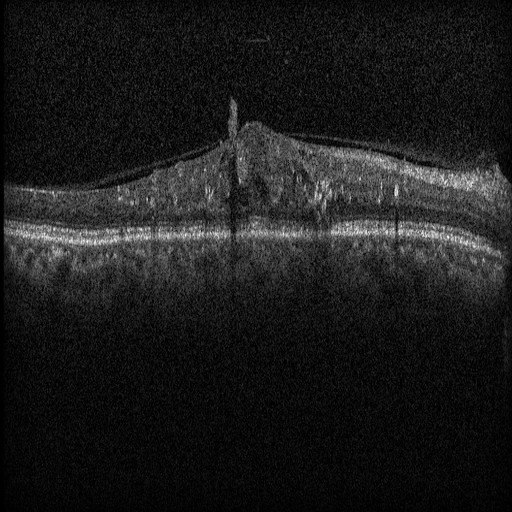

Optical coherence tomography scan. Finding: diabetic macular edema (DME).